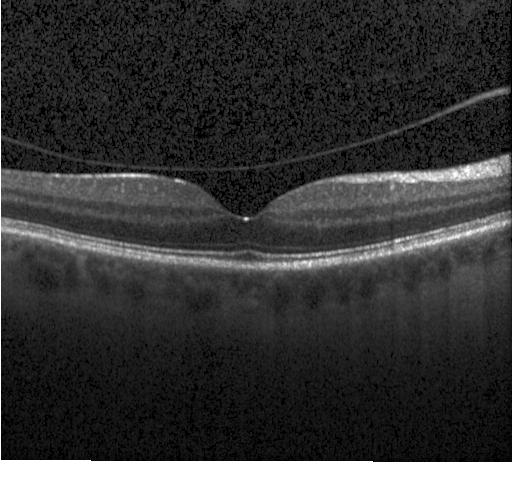 Instrument: Heidelberg Spectralis · fovea-centered · OCT B-scan
Impression: no choroidal neovascularization, no diabetic macular edema, and no drusen.